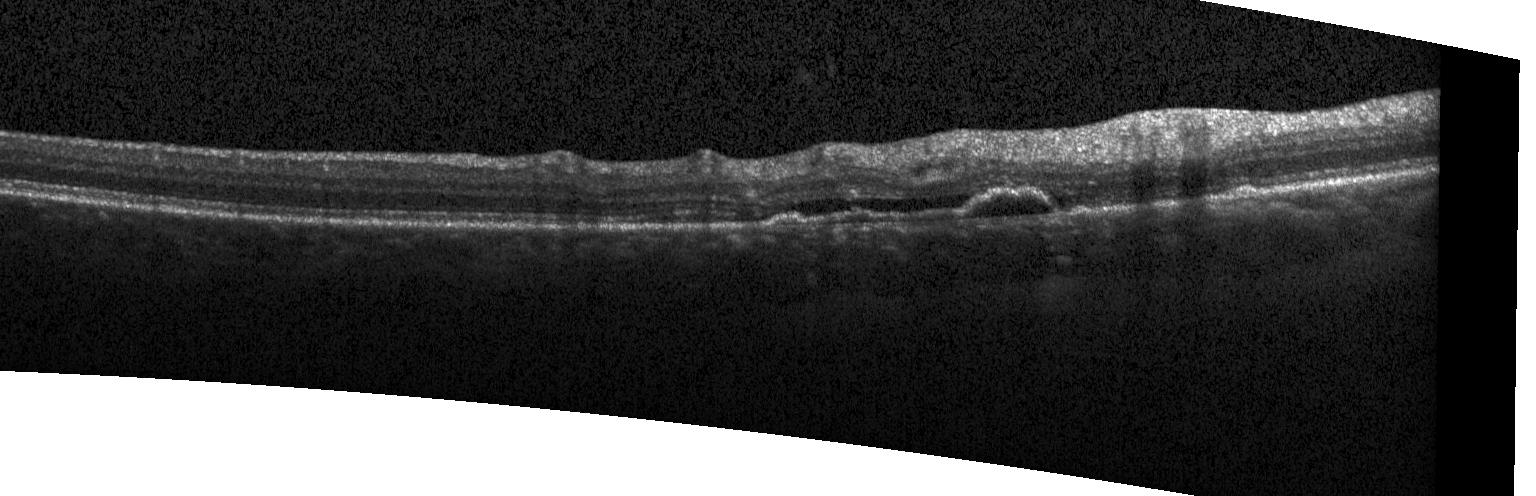
Finding: choroidal neovascularization.